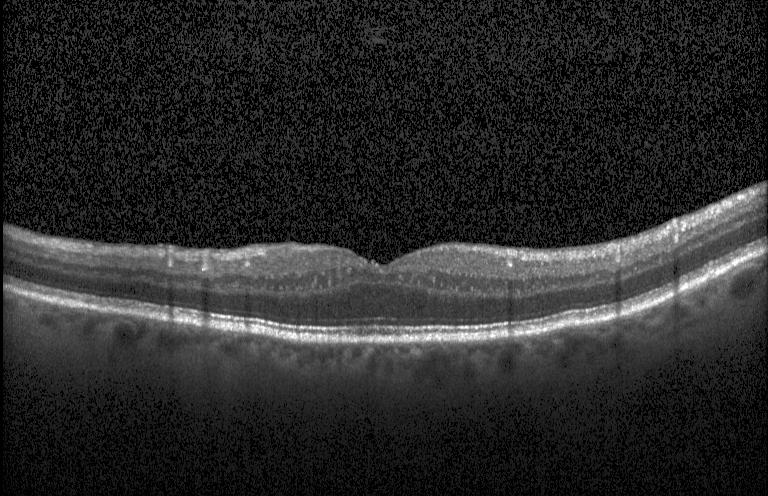

Retinal OCT B-scan — No evidence of choroidal neovascularization, diabetic macular edema, or drusen.